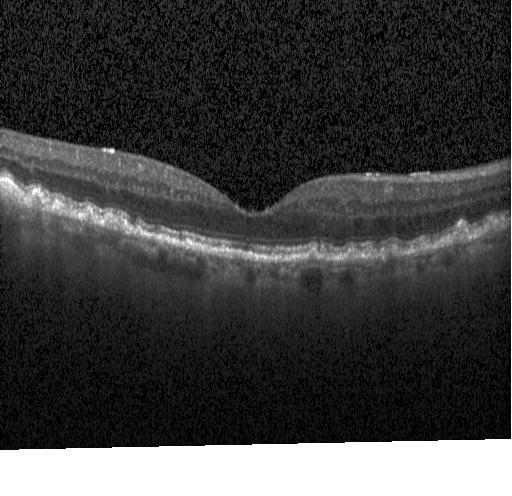 Finding: sub-RPE drusenoid deposits.